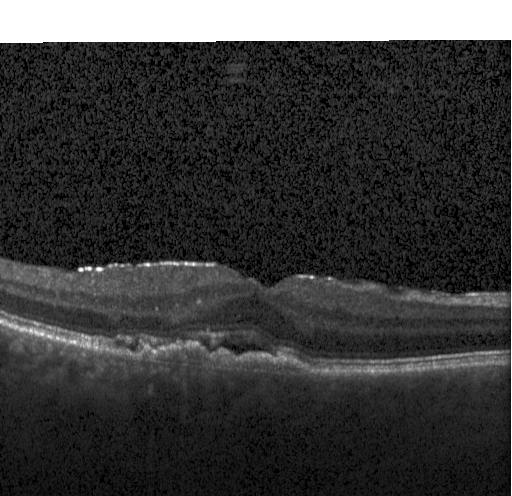
The scan shows a choroidal neovascular membrane.